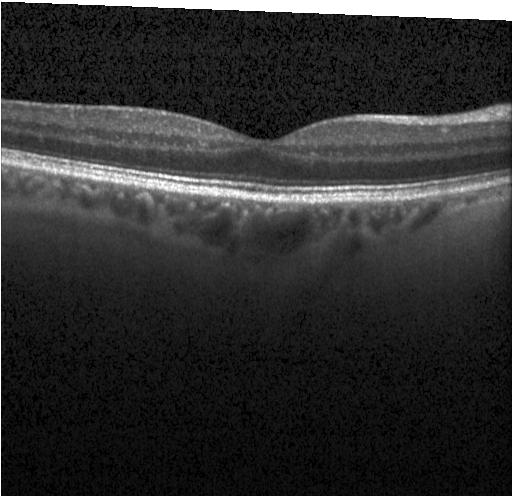

Spectral-domain optical coherence tomography; OCT line scan; instrument: Heidelberg Spectralis
Finding: no choroidal neovascularization, diabetic macular edema, or drusen.